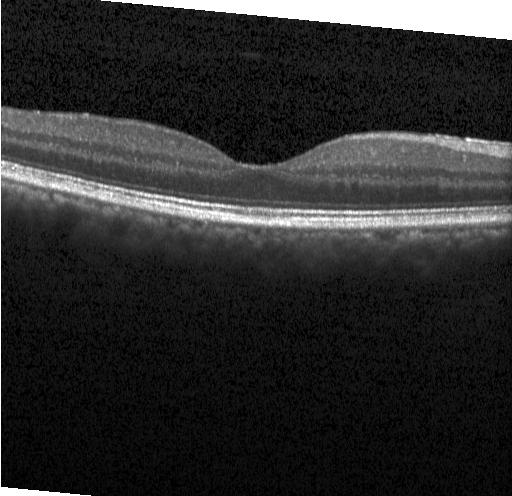

Macular OCT demonstrating no choroidal neovascularization, no diabetic macular edema, and no drusen.